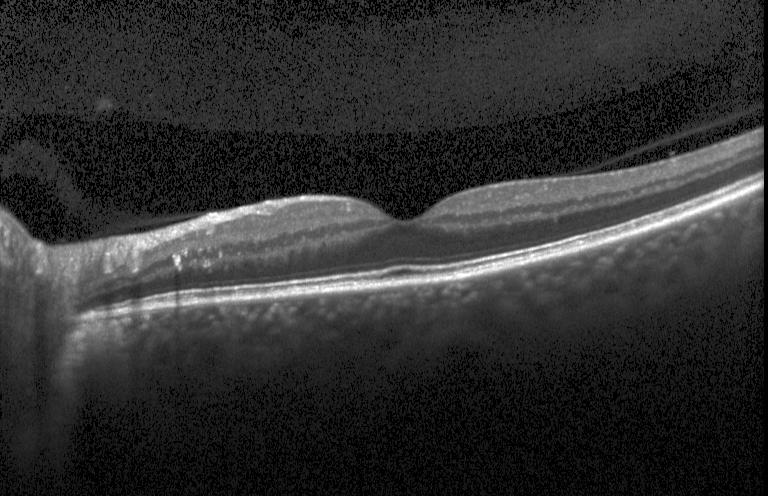 Diagnosis: no choroidal neovascularization, no diabetic macular edema, and no drusen.